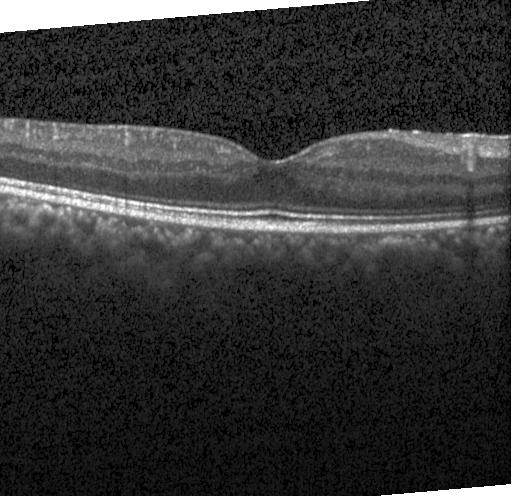
OCT B-scan showing no choroidal neovascularization, no diabetic macular edema, and no drusen.